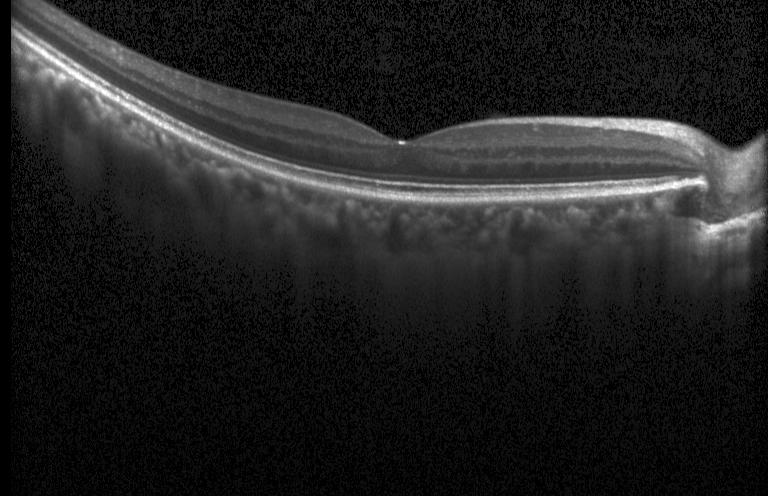 Macular scan · retinal OCT cross-section
Macular OCT: no CNV, no DME, and no drusen.